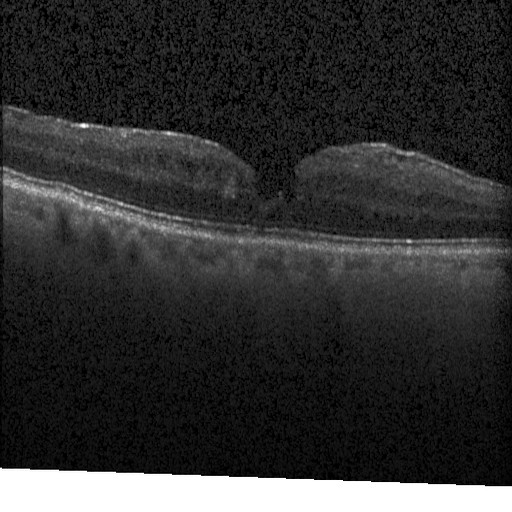

Macular OCT demonstrating diabetic macular edema.